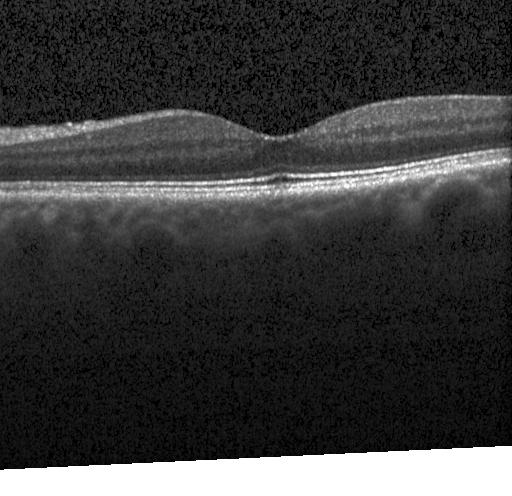

Impression: no CNV, no DME, and no drusen.